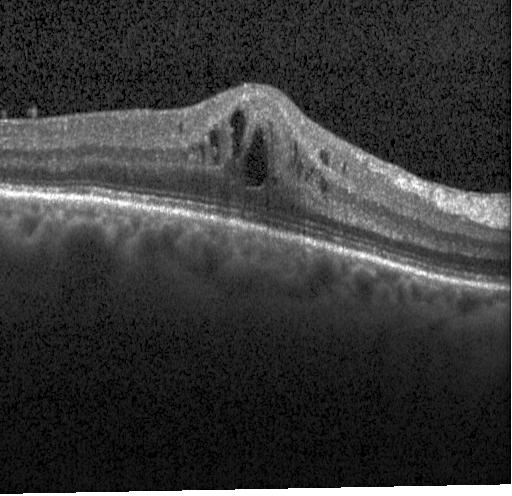
Diagnosis: DME.